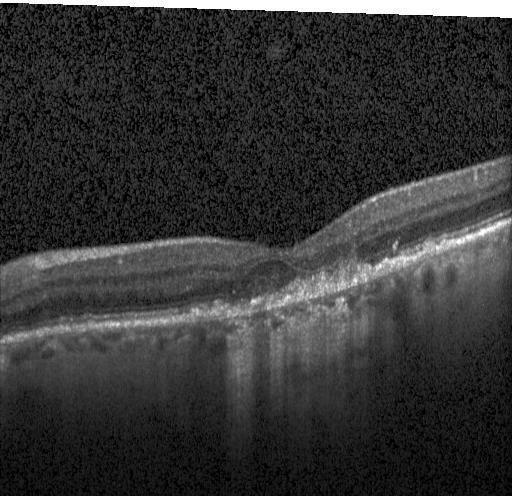
Diagnosis: a choroidal neovascular membrane.